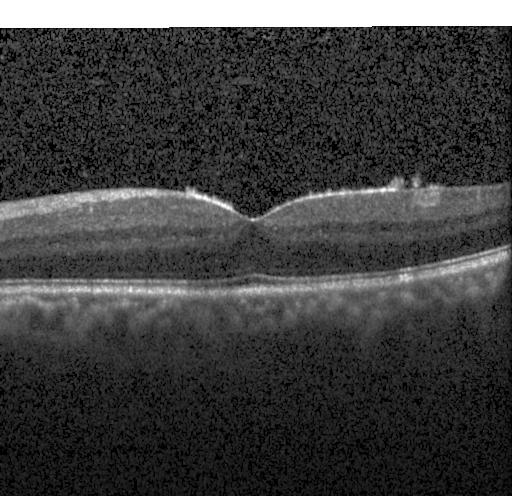

Optical coherence tomography scan. Diagnosis: no choroidal neovascularization, no diabetic macular edema, and no drusen.